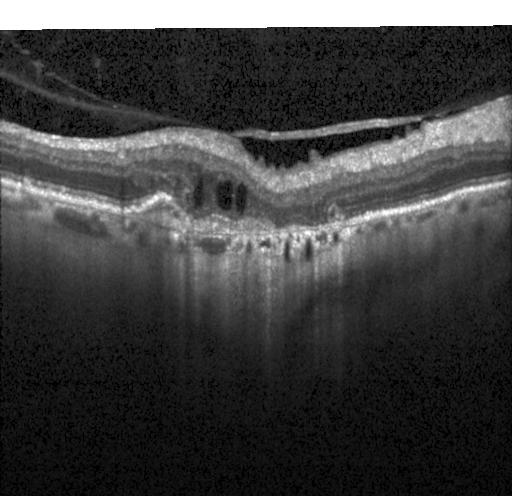
Dx: CNV.